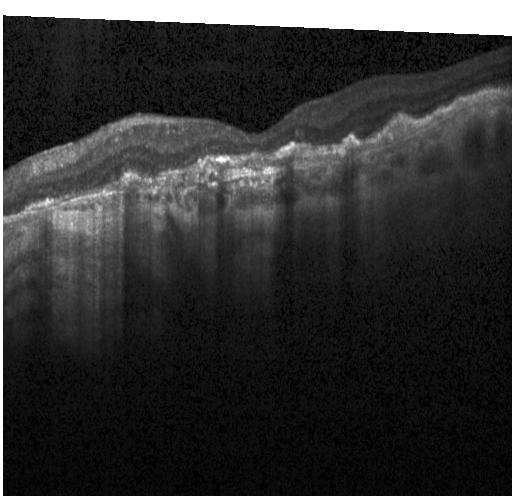

OCT B-scan — Macular OCT: a choroidal neovascular membrane.